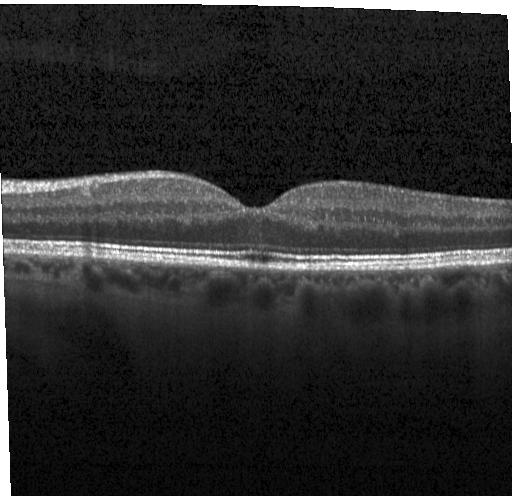
Retinal OCT B-scan. The scan shows no choroidal neovascularization, no diabetic macular edema, and no drusen.